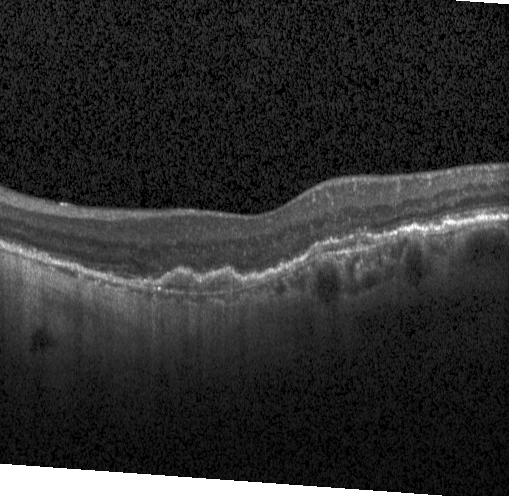

Retinal OCT cross-section · through the macula. Macular OCT: choroidal neovascularization.